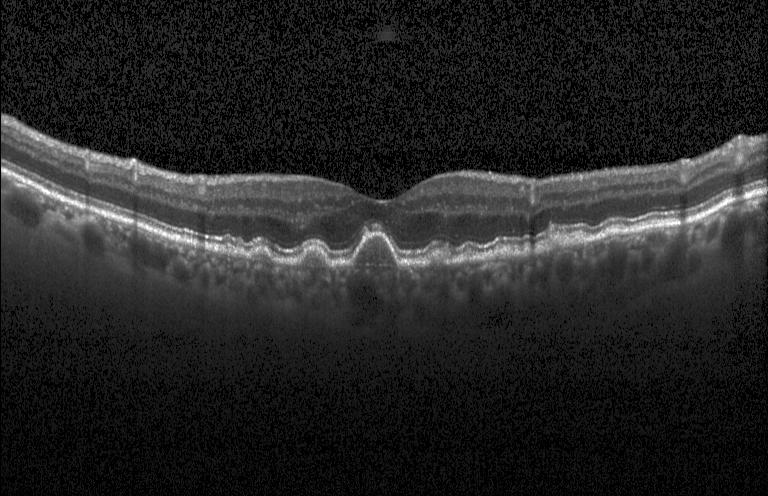
SD-OCT. Heidelberg Spectralis. Horizontal scan through the fovea. Optical coherence tomography scan. The scan shows multiple drusen.